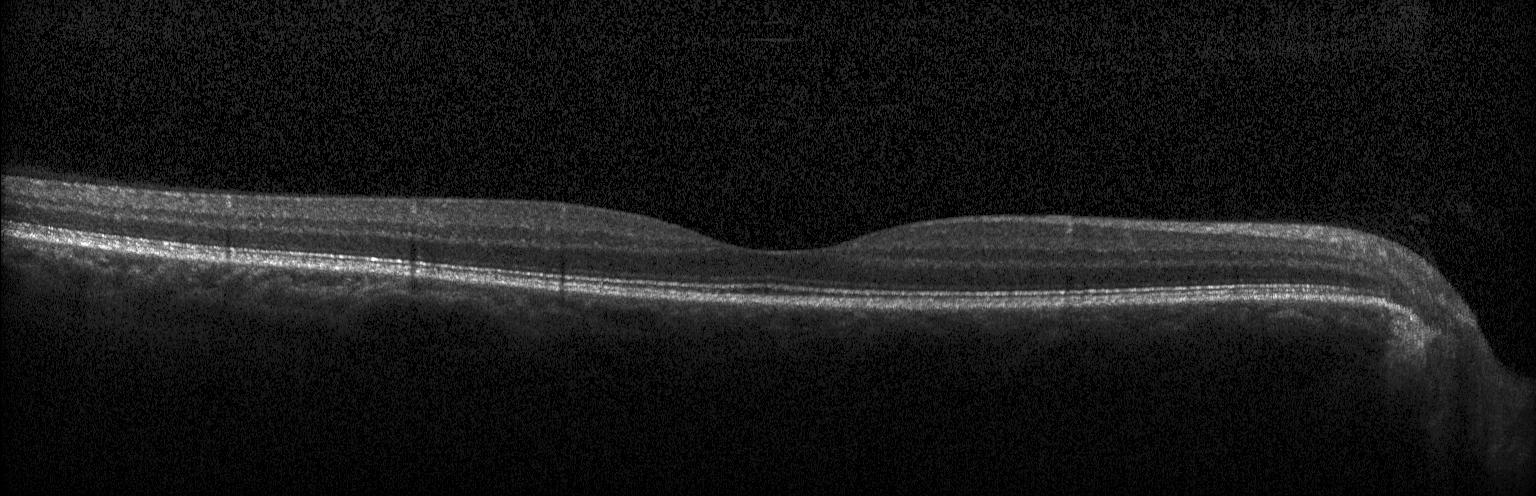

OCT line scan — OCT finding: no evidence of choroidal neovascularization, diabetic macular edema, or drusen.